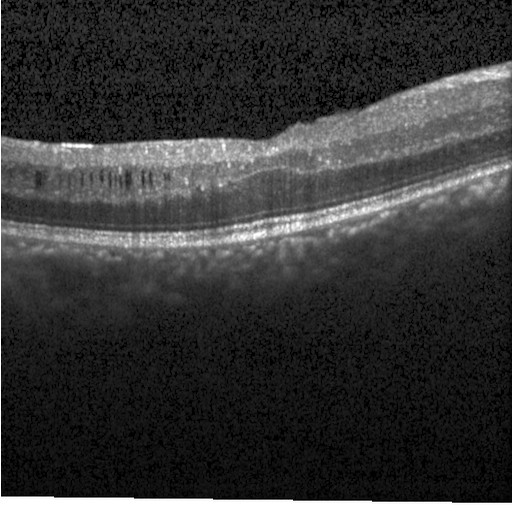
Macular OCT demonstrating diabetic macular edema.